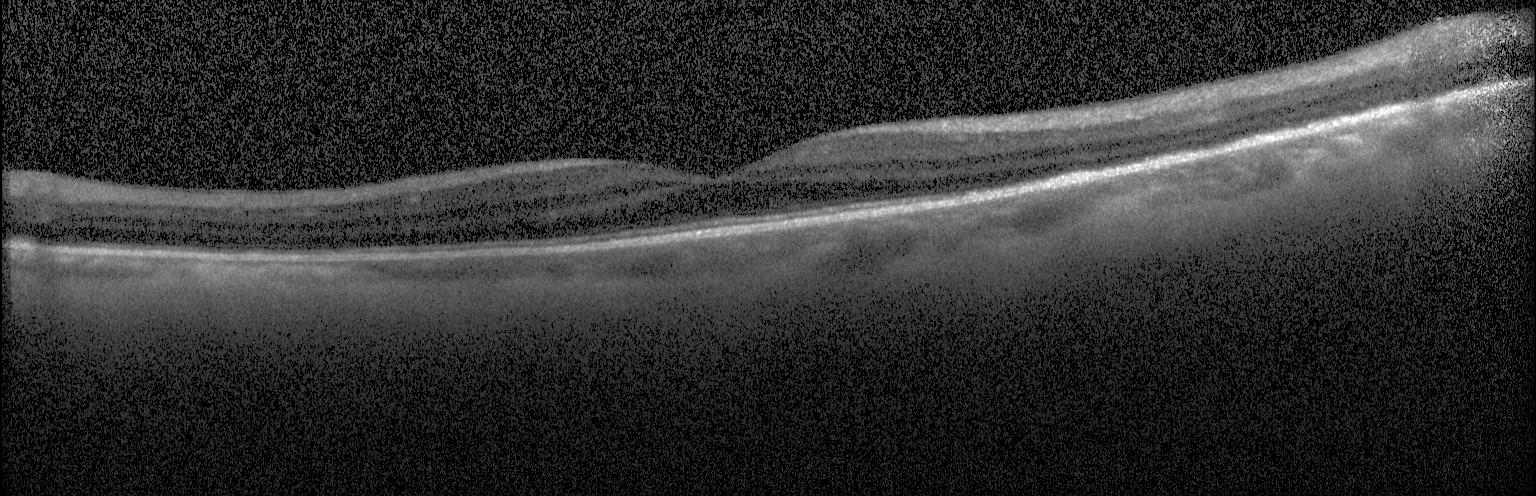
Macular OCT demonstrating no choroidal neovascularization, diabetic macular edema, or drusen.